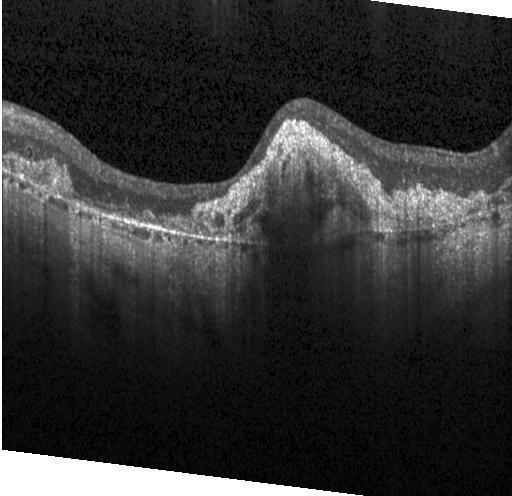

Finding: choroidal neovascularization (CNV).